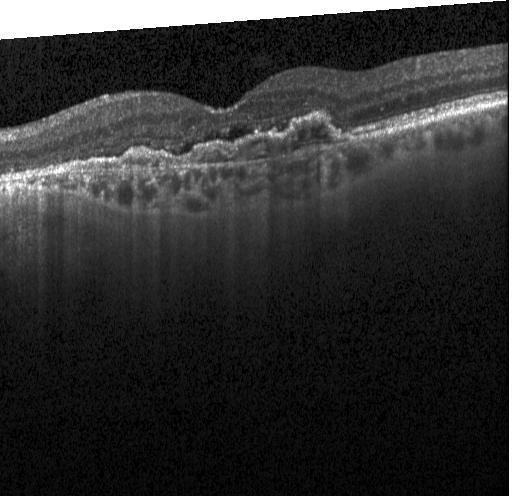

Diagnosis: CNV.